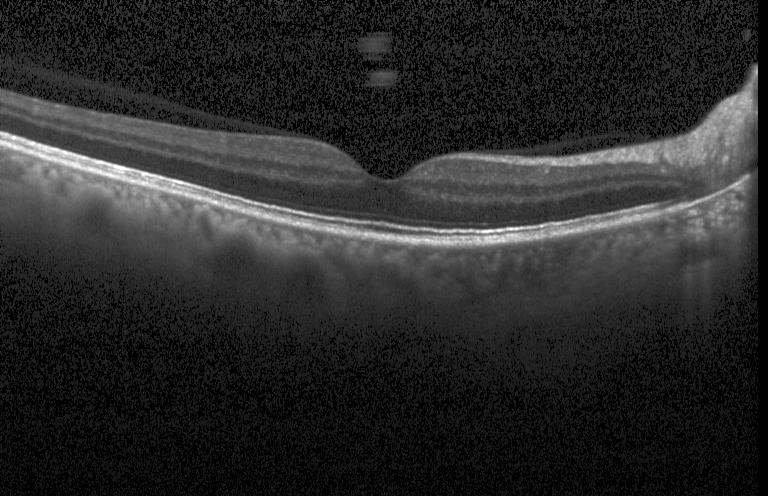 Spectral-domain optical coherence tomography; OCT line scan; through the macula. Finding: no CNV, no DME, and no drusen.